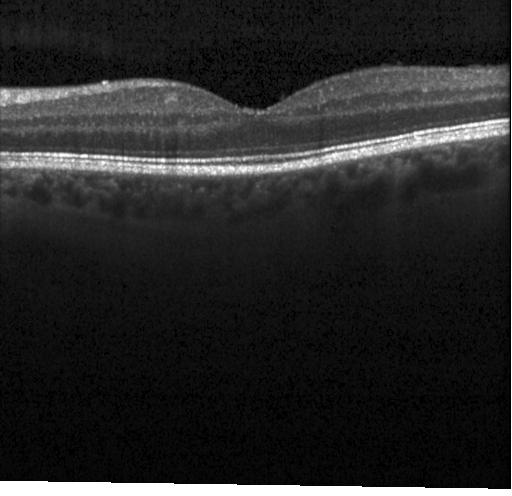
OCT B-scan showing no choroidal neovascularization, no diabetic macular edema, and no drusen.